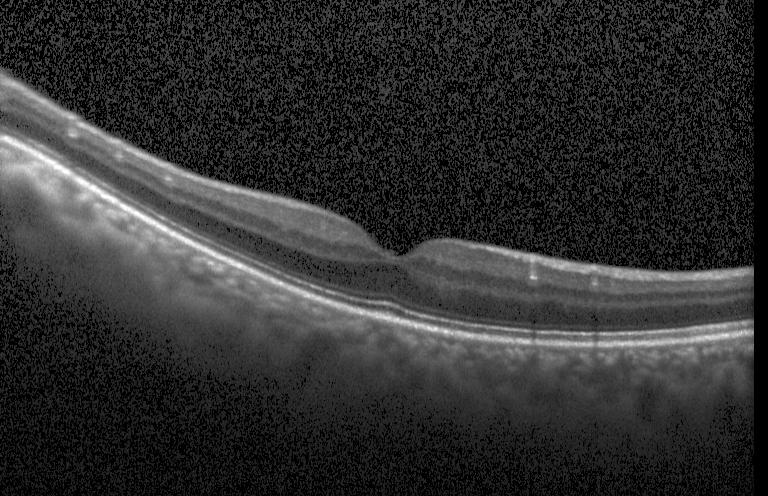 Retinal OCT cross-section — Finding: neither choroidal neovascularization, diabetic macular edema, nor drusen.